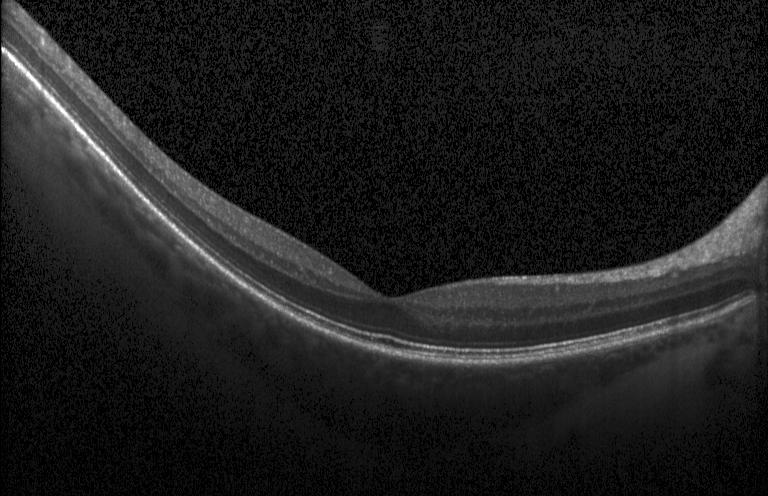 Optical coherence tomography scan, instrument: Heidelberg Spectralis
Finding: no evidence of CNV, DME, or drusen.